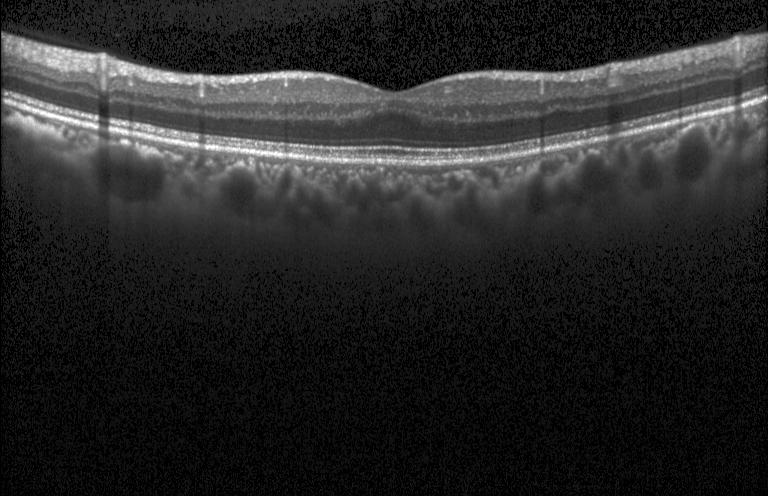

OCT B-scan; centered on the fovea; instrument: Heidelberg Spectralis; spectral-domain OCT.
Macular OCT: neither choroidal neovascularization, diabetic macular edema, nor drusen.